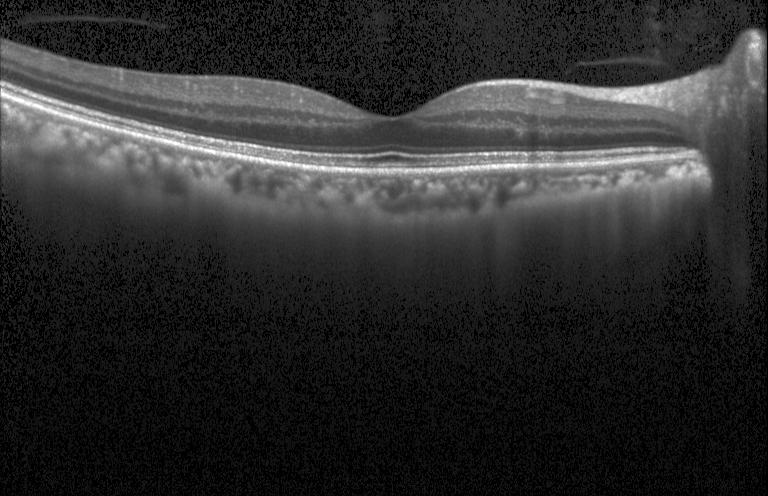

Retinal OCT B-scan; horizontal scan through the fovea — This B-scan demonstrates no evidence of choroidal neovascularization, diabetic macular edema, or drusen.